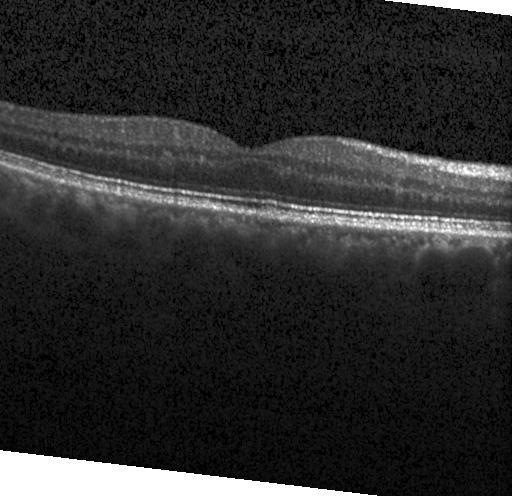
OCT finding: no CNV, no DME, and no drusen.